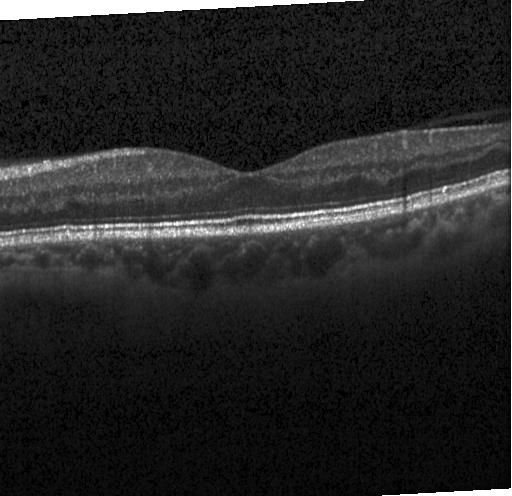 Retinal OCT cross-section · macular scan.
Assessment: no choroidal neovascularization, no diabetic macular edema, and no drusen.